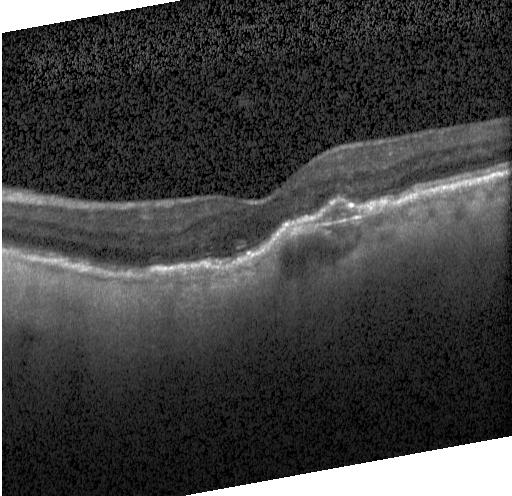 Spectral-domain optical coherence tomography. OCT B-scan.
OCT finding: CNV.